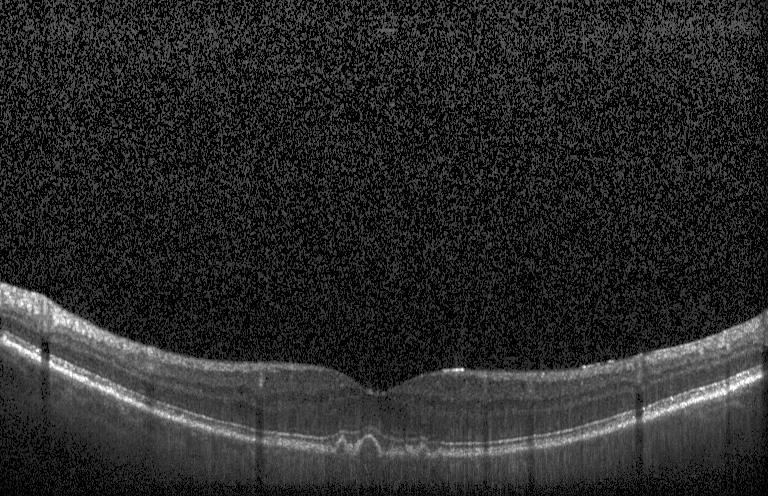

Spectral-domain OCT. Heidelberg Spectralis. OCT B-scan
Assessment: drusen.